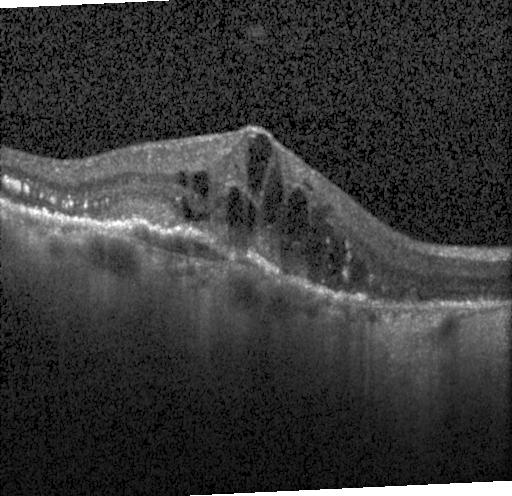
Optical coherence tomography scan, macular scan.
The scan shows choroidal neovascularization (CNV).